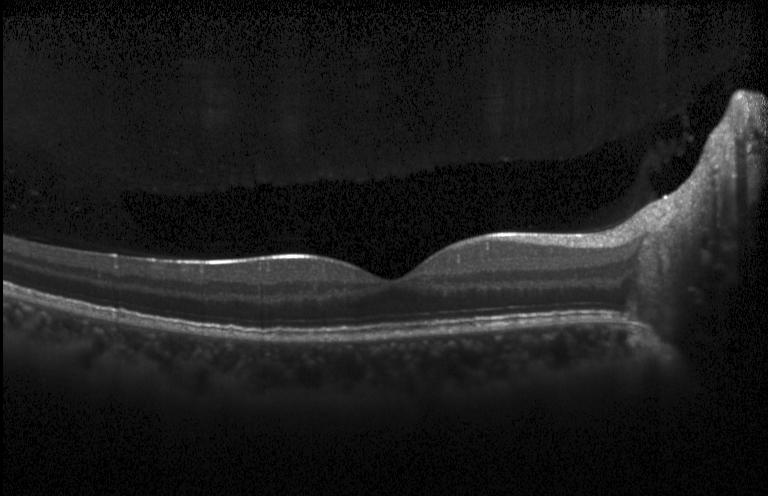

Retinal OCT B-scan
Impression: no CNV, DME, or drusen.